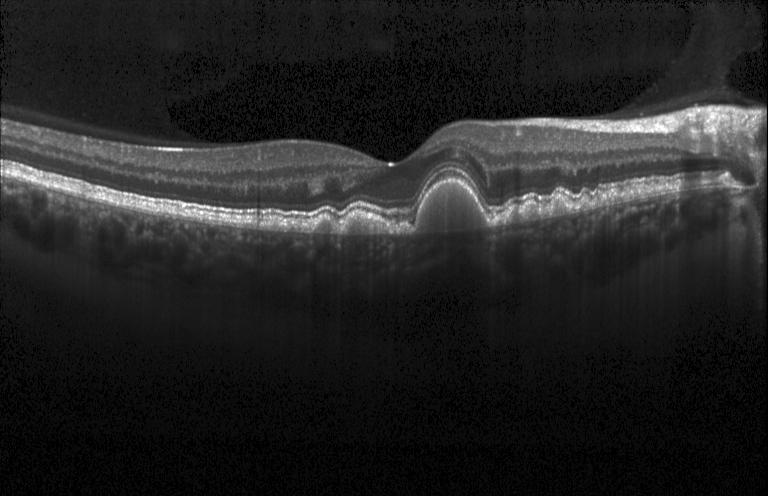 Dx: multiple drusen.